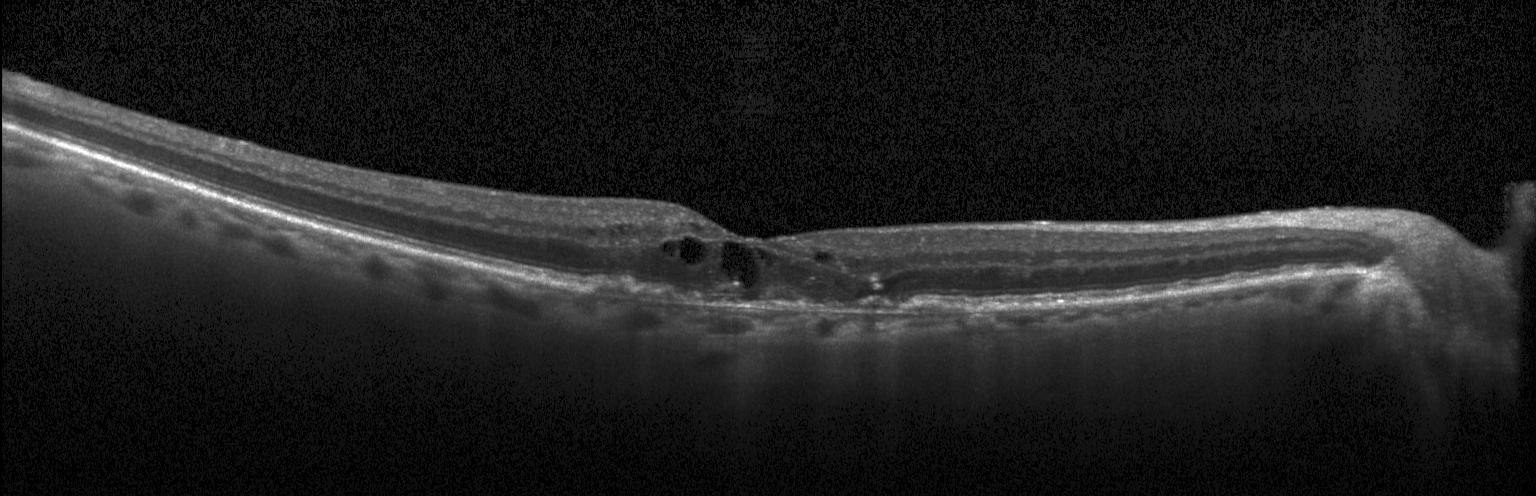
OCT line scan, Heidelberg Spectralis OCT system, SD-OCT. Dx: a choroidal neovascular membrane.